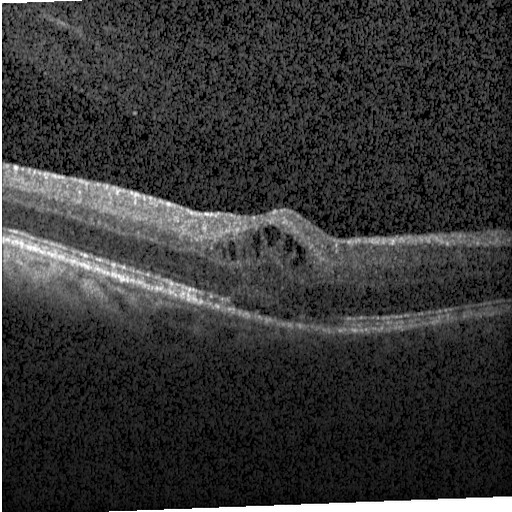

OCT line scan
Dx: diabetic macular edema (DME).